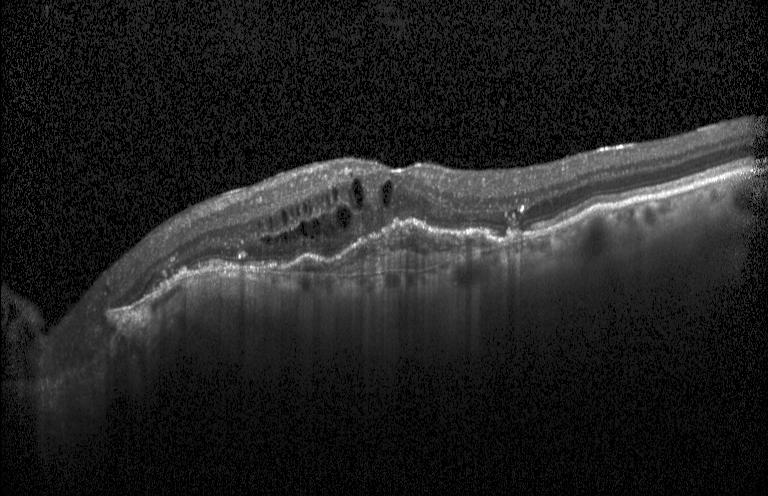 Acquired on a Heidelberg Spectralis; macular scan; spectral-domain OCT; retinal OCT cross-section — CNV.